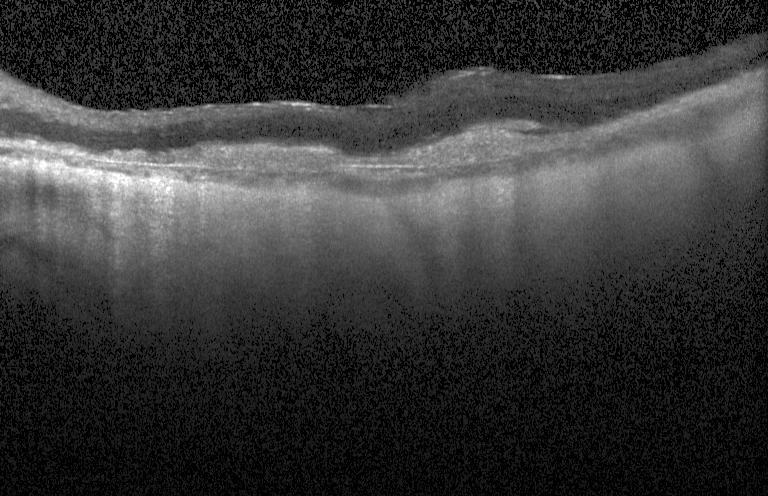

SD-OCT · optical coherence tomography B-scan · centered on the fovea · instrument: Heidelberg Spectralis
Finding: choroidal neovascularization.